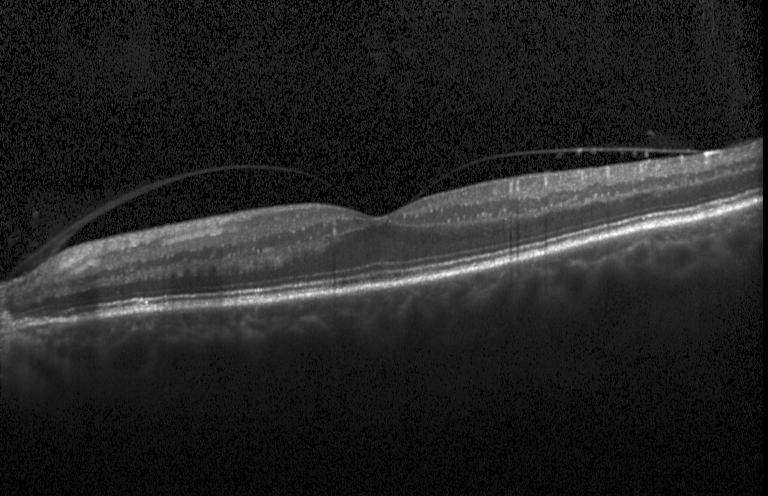
Macular scan, optical coherence tomography scan
Neither choroidal neovascularization, diabetic macular edema, nor drusen.